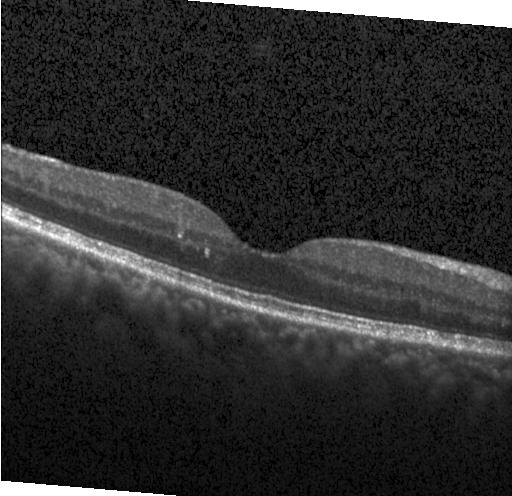
Fovea-centered; retinal OCT cross-section.
Diagnosis: no choroidal neovascularization, no diabetic macular edema, and no drusen.